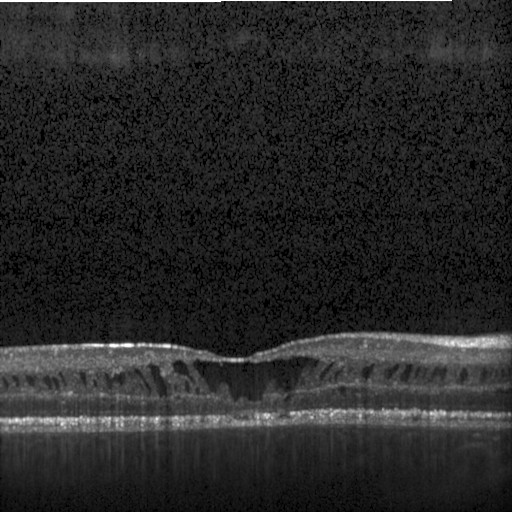 Impression: diabetic macular edema (DME).